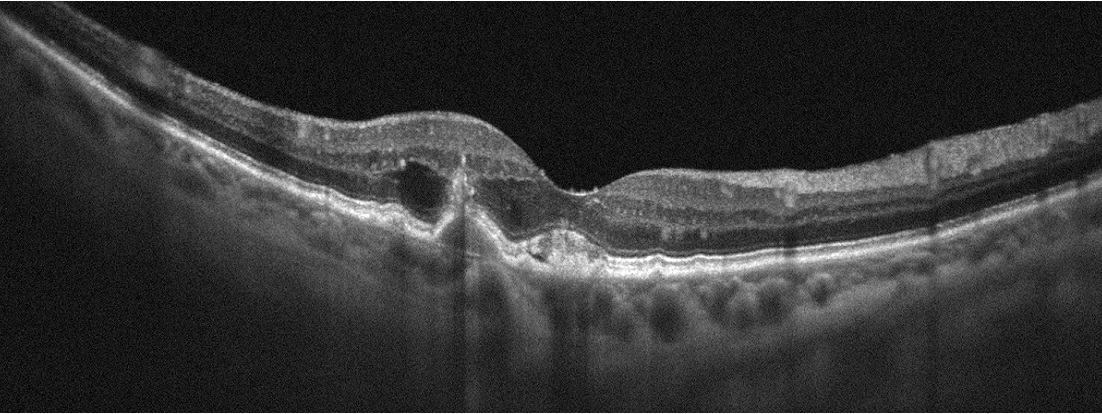
Assessment: age-related macular degeneration (AMD).